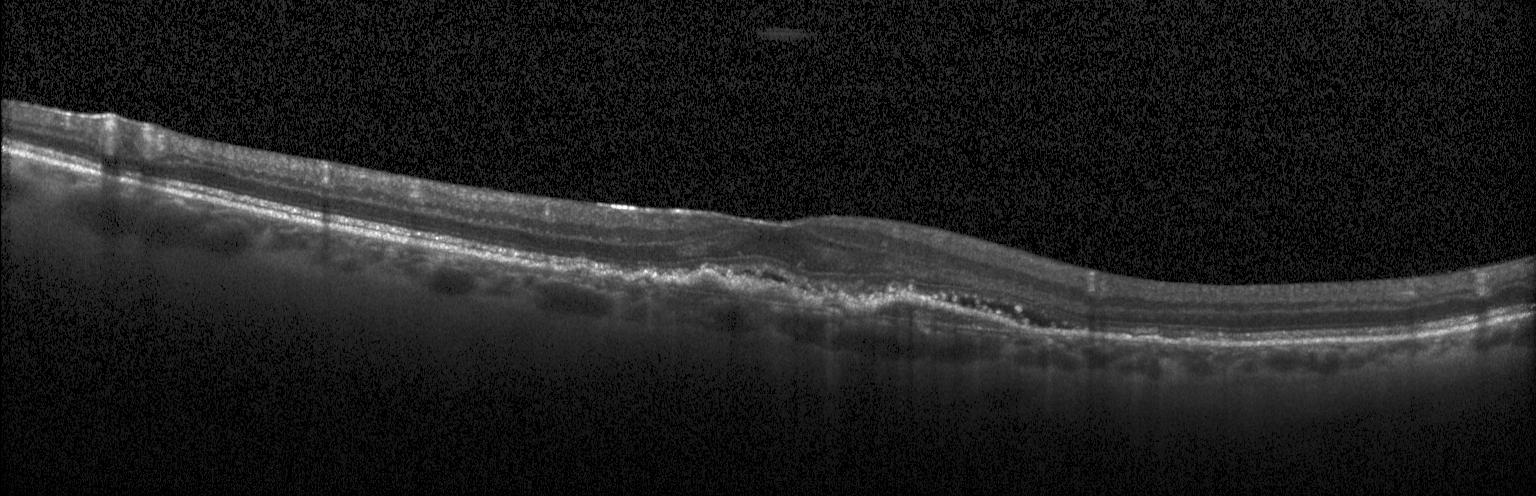
OCT finding: a choroidal neovascular membrane.